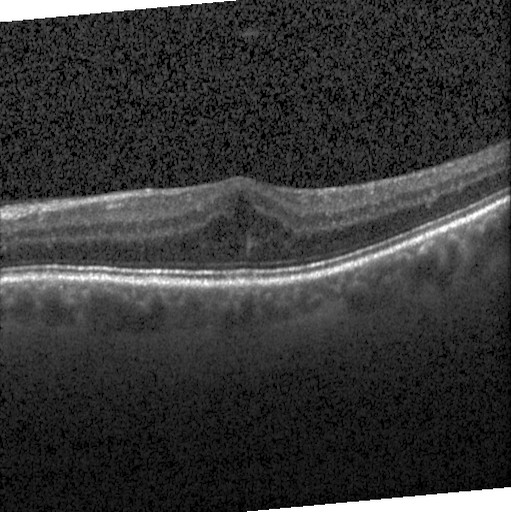 Finding: DME.